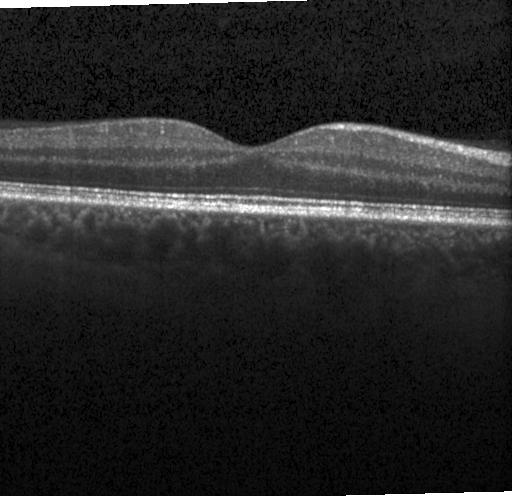

Instrument: Heidelberg Spectralis, spectral-domain optical coherence tomography, optical coherence tomography B-scan.
Finding: no CNV, DME, or drusen.